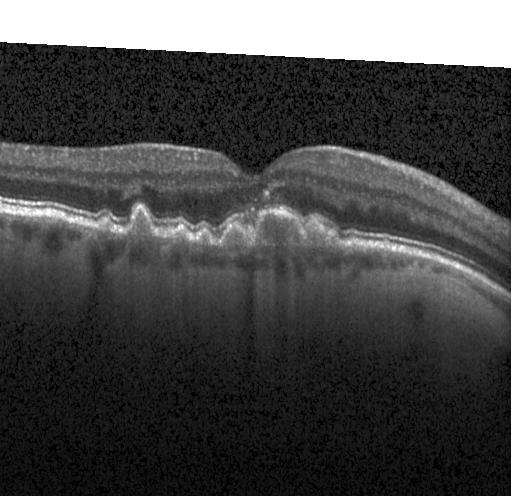

Through the macula. Heidelberg Spectralis OCT system. Optical coherence tomography scan. Spectral-domain OCT
This B-scan demonstrates multiple drusen.